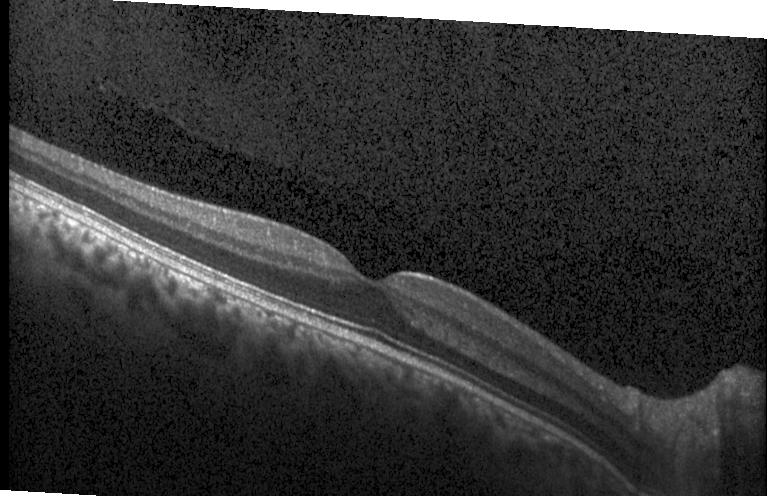
Diagnosis: no evidence of choroidal neovascularization, diabetic macular edema, or drusen.